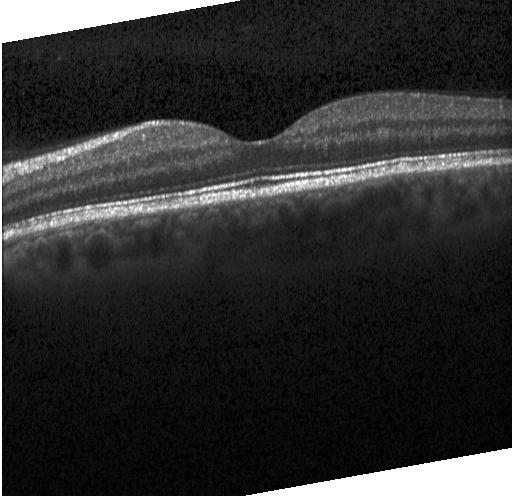 Impression: no CNV, no DME, and no drusen.